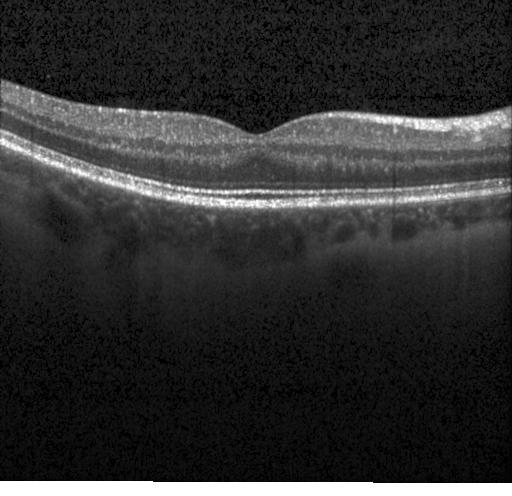 Retinal OCT cross-section; spectral-domain optical coherence tomography. Dx: no evidence of choroidal neovascularization, diabetic macular edema, or drusen.